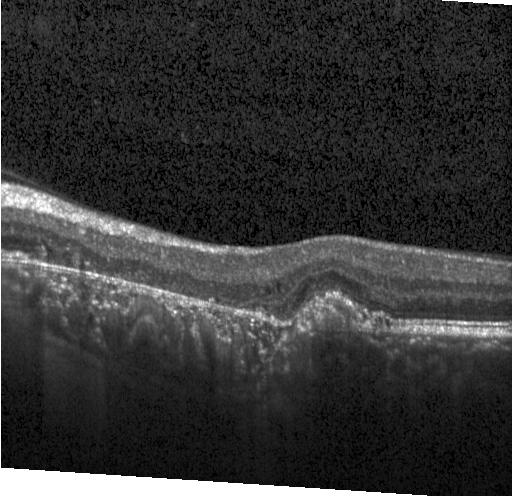

Spectral-domain OCT. Heidelberg Spectralis. OCT B-scan. Dx: a choroidal neovascular membrane.